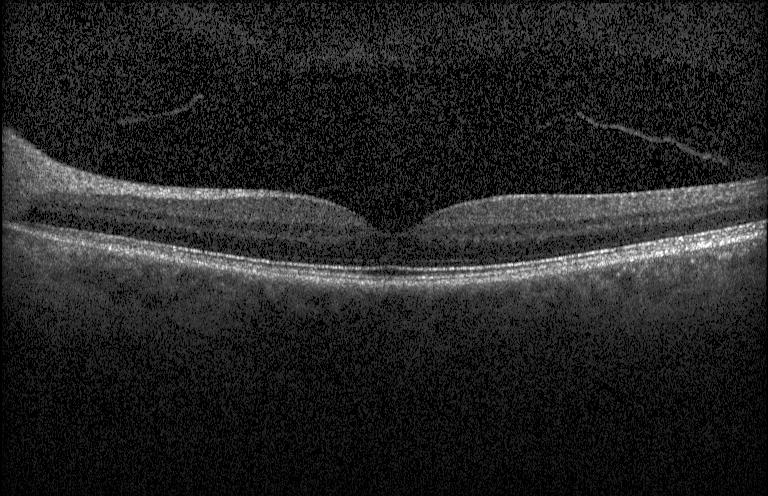 Impression: no choroidal neovascularization, diabetic macular edema, or drusen.